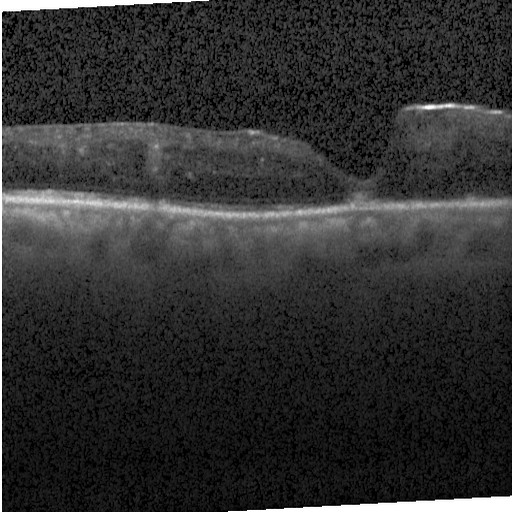
Macular OCT demonstrating diabetic macular edema (DME).